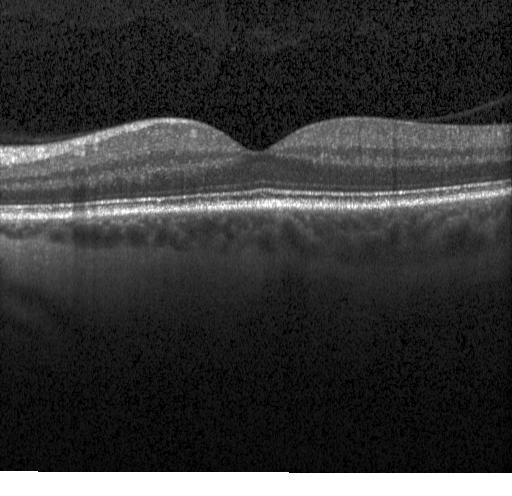

Horizontal scan through the fovea; spectral-domain optical coherence tomography; Heidelberg Spectralis; OCT B-scan. Dx: no choroidal neovascularization, no diabetic macular edema, and no drusen.